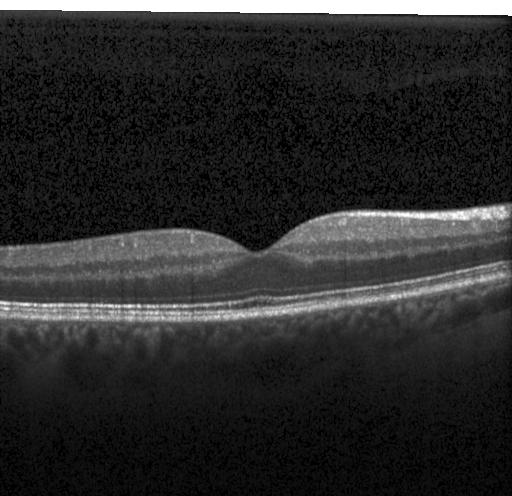
Centered on the fovea, retinal OCT B-scan, spectral-domain optical coherence tomography, instrument: Heidelberg Spectralis. The scan shows neither CNV, DME, nor drusen.